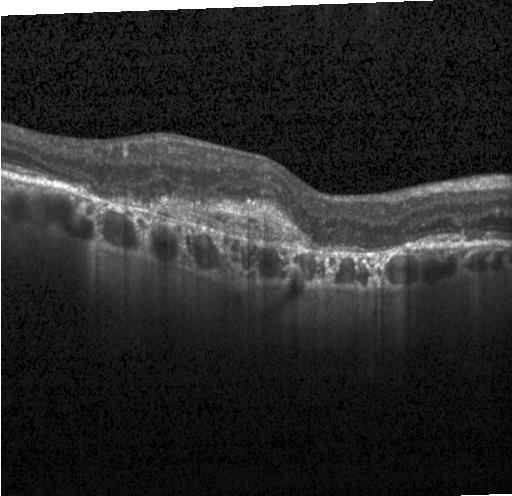

OCT B-scan — Impression: a choroidal neovascular membrane.